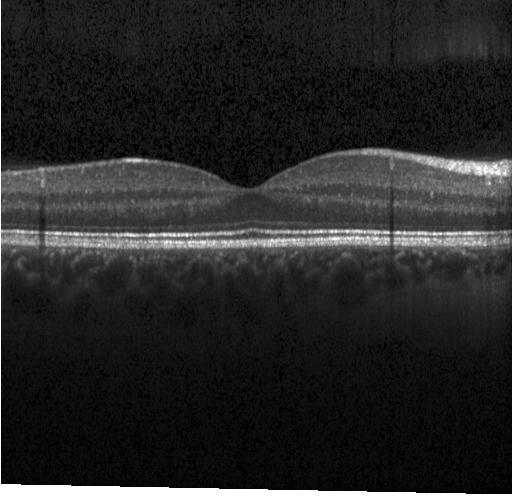

Finding: no CNV, DME, or drusen.